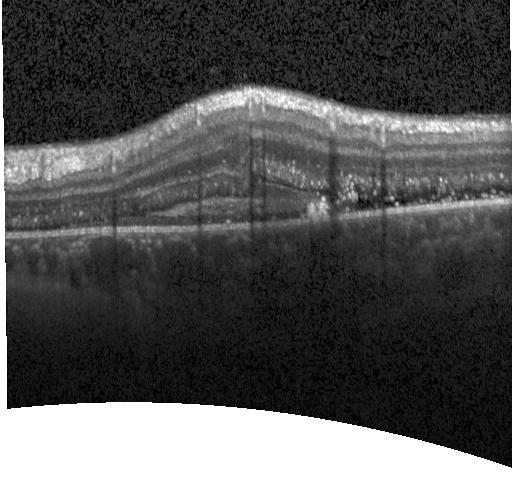 Retinal OCT B-scan. Heidelberg Spectralis OCT system. Through the macula.
Finding: choroidal neovascularization (CNV).